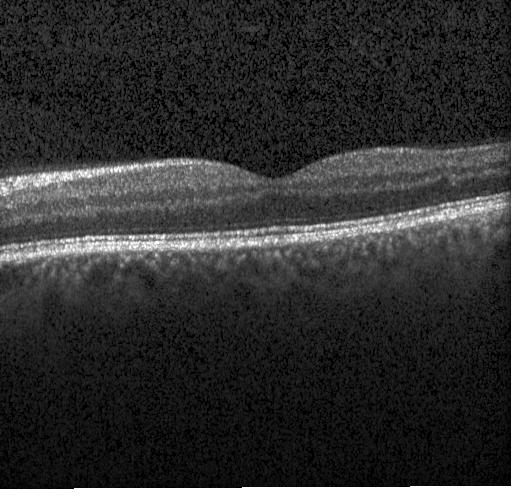
Horizontal scan through the fovea · instrument: Heidelberg Spectralis · OCT line scan. Neither choroidal neovascularization, diabetic macular edema, nor drusen.